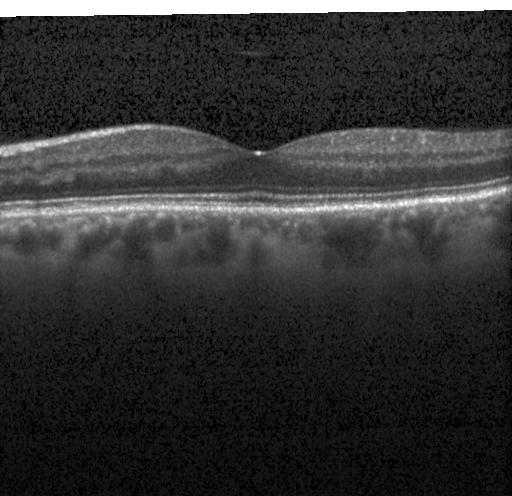 Dx: no choroidal neovascularization, no diabetic macular edema, and no drusen.